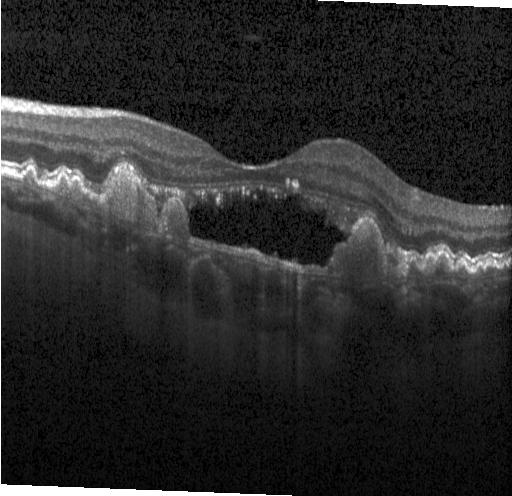

OCT finding: a choroidal neovascular membrane.